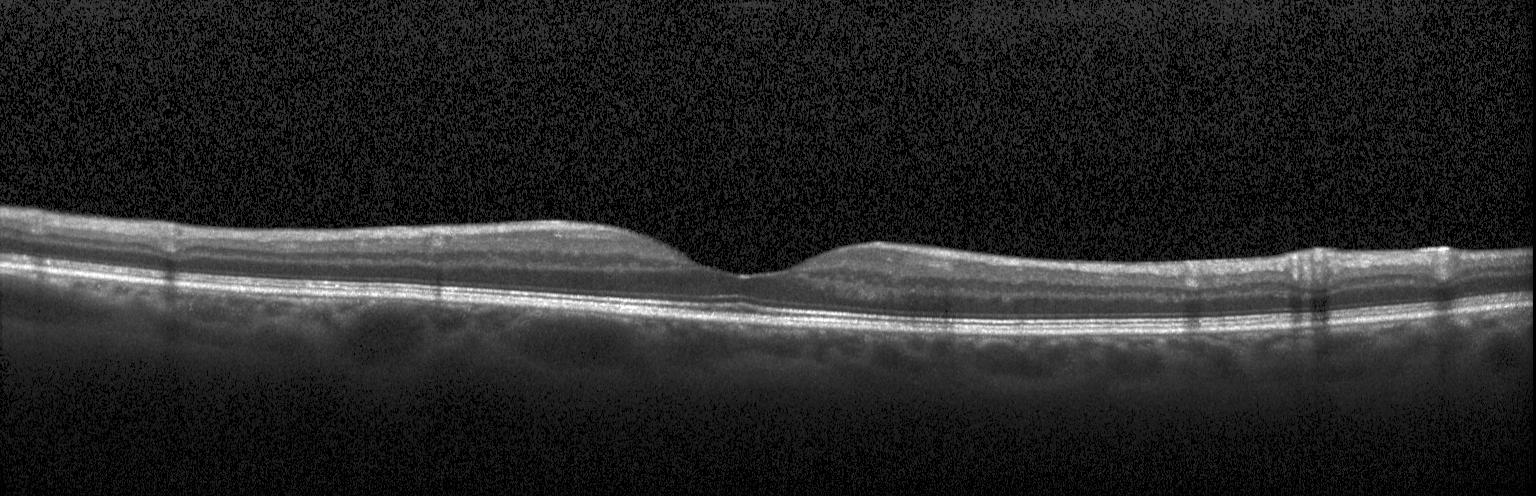
OCT B-scan showing no choroidal neovascularization, no diabetic macular edema, and no drusen.